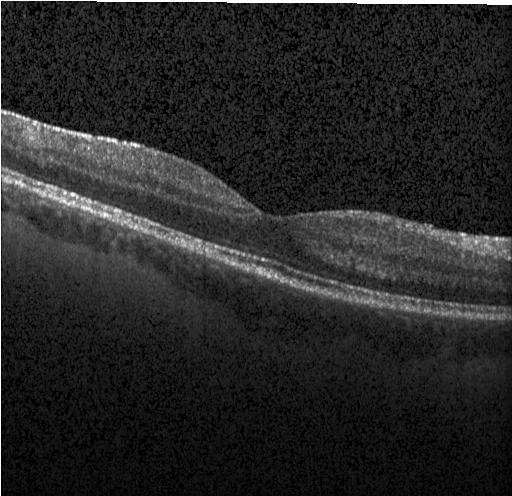

Fovea-centered · Heidelberg Spectralis · optical coherence tomography scan · SD-OCT — Diagnosis: neither CNV, DME, nor drusen.